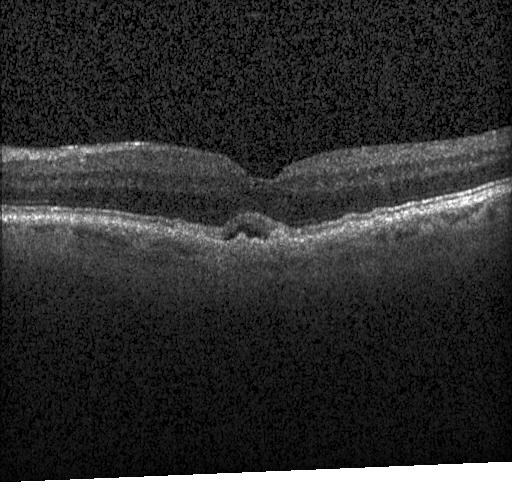
Finding: choroidal neovascularization.